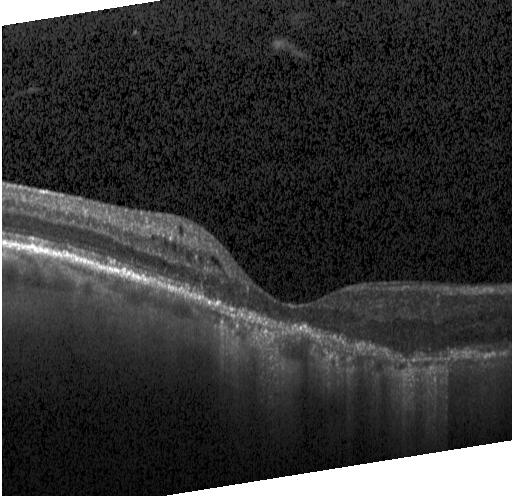
Optical coherence tomography B-scan — Diagnosis: choroidal neovascularization.